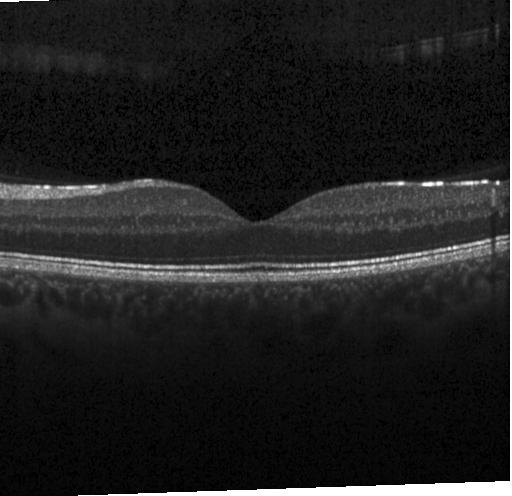
OCT B-scan · horizontal scan through the fovea · spectral-domain OCT
OCT finding: no CNV, DME, or drusen.